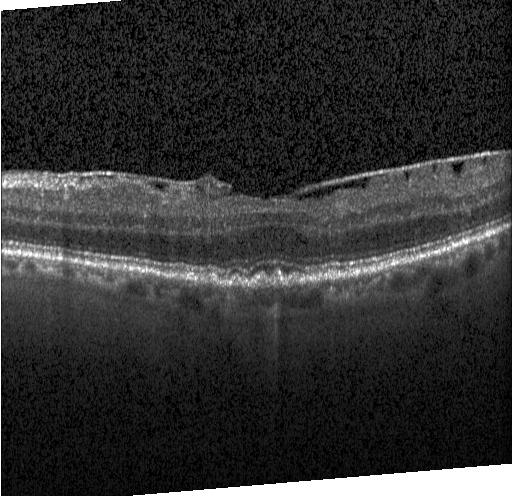 OCT line scan; SD-OCT.
Assessment: drusen.